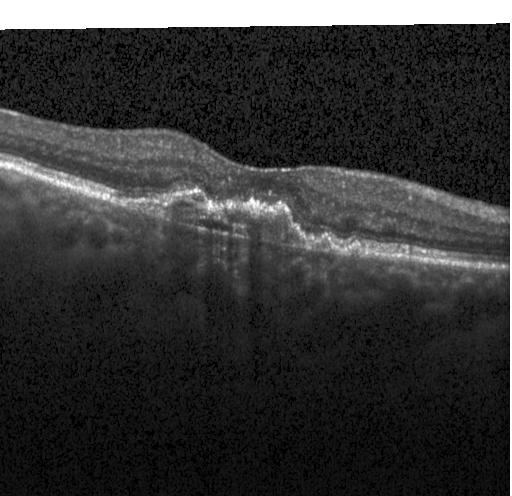
Optical coherence tomography scan · horizontal scan through the fovea.
Impression: choroidal neovascularization (CNV).